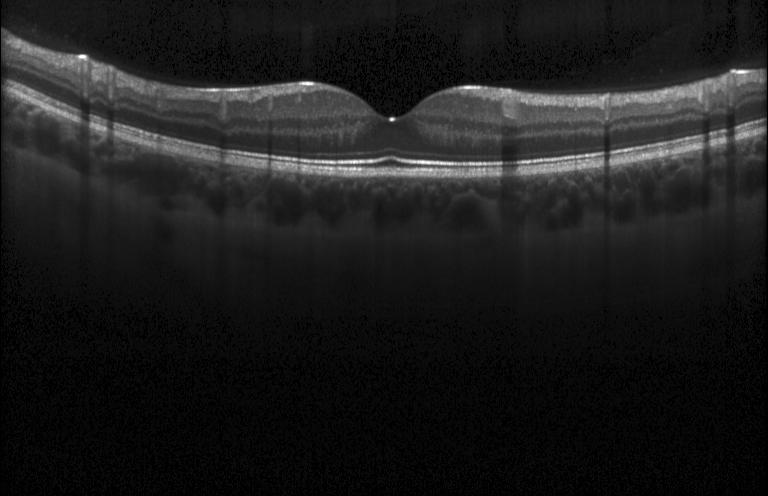
Spectral-domain optical coherence tomography. Centered on the fovea. Retinal OCT cross-section. Acquired on a Heidelberg Spectralis
This B-scan demonstrates no choroidal neovascularization, diabetic macular edema, or drusen.